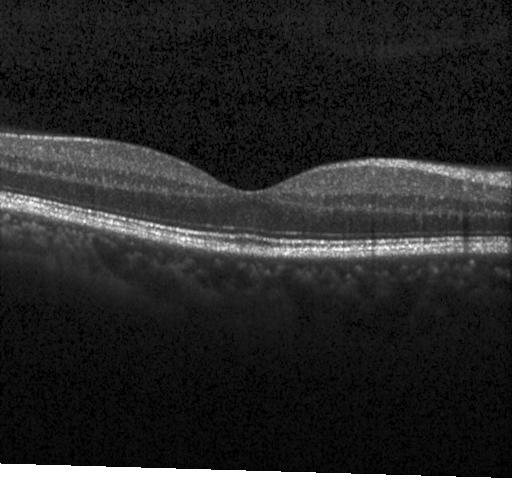 OCT B-scan showing no CNV, DME, or drusen.